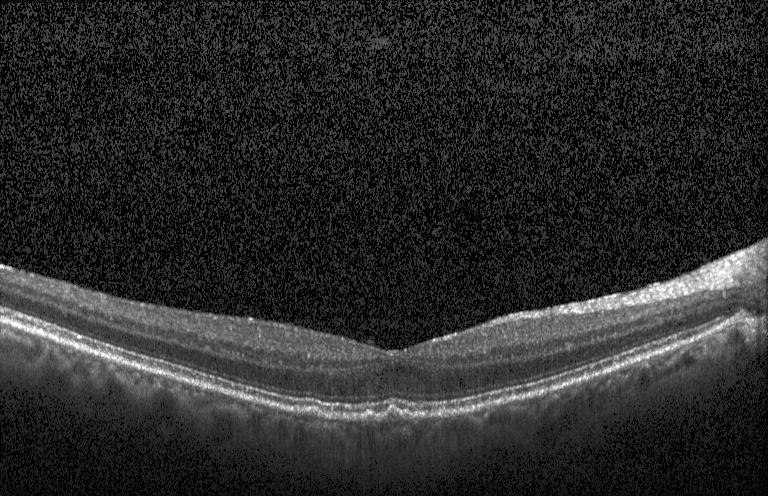 Through the macula. SD-OCT. Optical coherence tomography scan. Heidelberg Spectralis OCT system.
Assessment: sub-RPE drusenoid deposits.